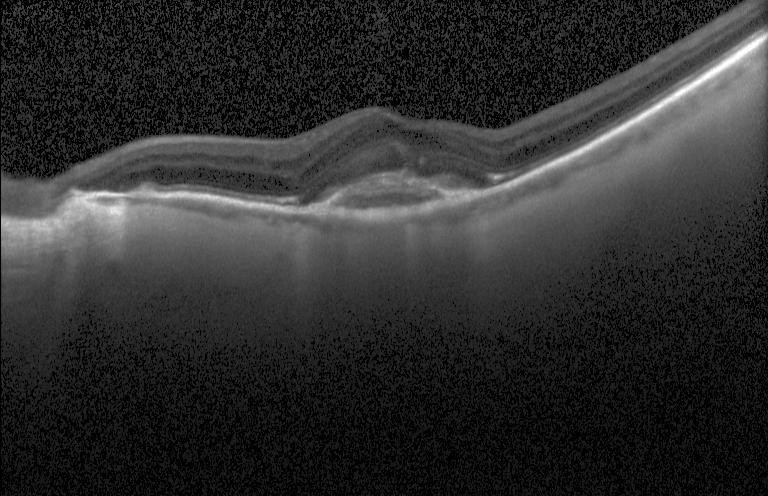

OCT line scan. Fovea-centered
Finding: a choroidal neovascular membrane.